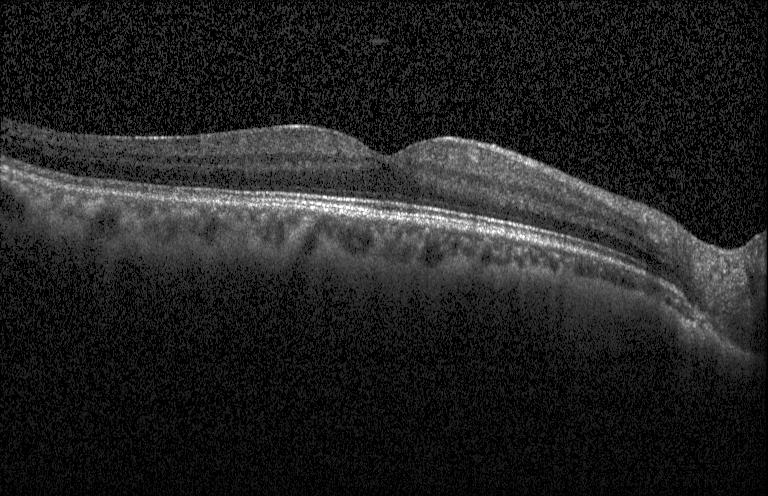 This B-scan demonstrates neither choroidal neovascularization, diabetic macular edema, nor drusen.